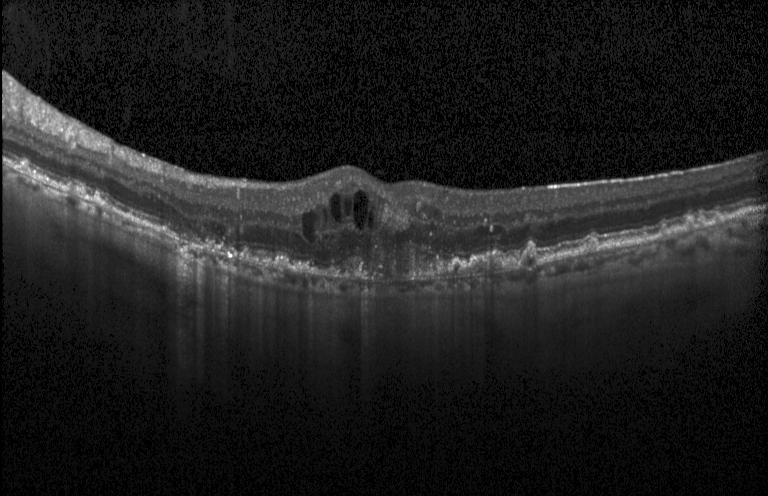

CNV.